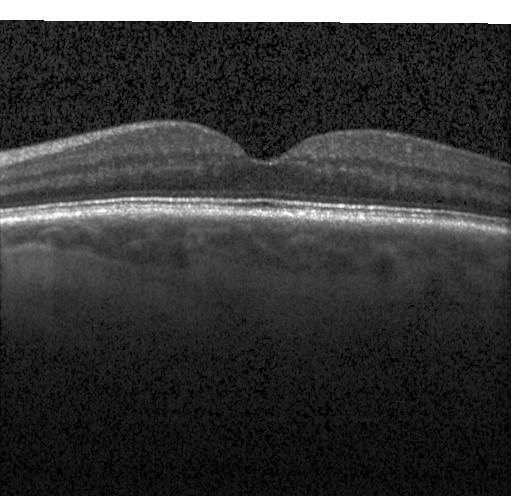 Optical coherence tomography scan.
Macular OCT: no CNV, no DME, and no drusen.